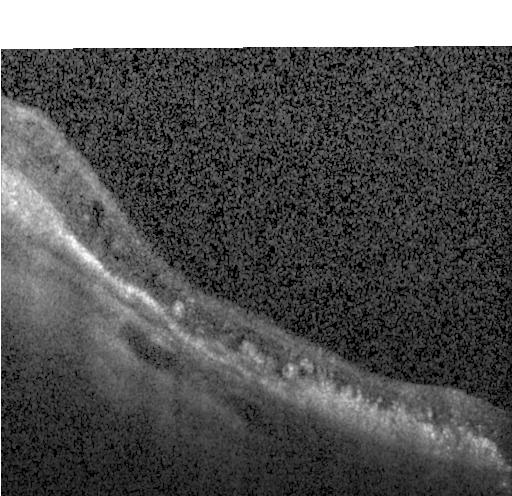
Through the macula · optical coherence tomography scan · spectral-domain OCT — Diagnosis: choroidal neovascularization.